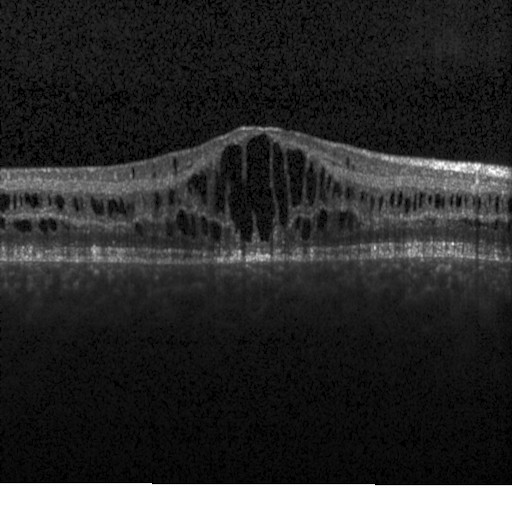

Spectral-domain OCT B-scan: DME.